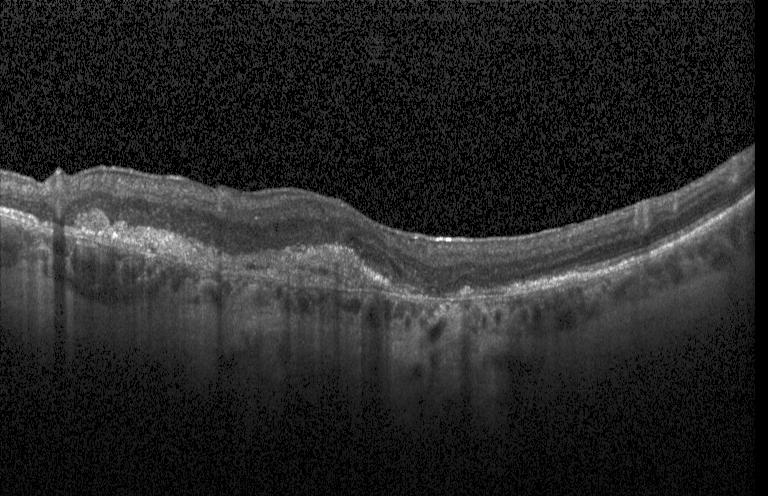

Macular OCT: a choroidal neovascular membrane.